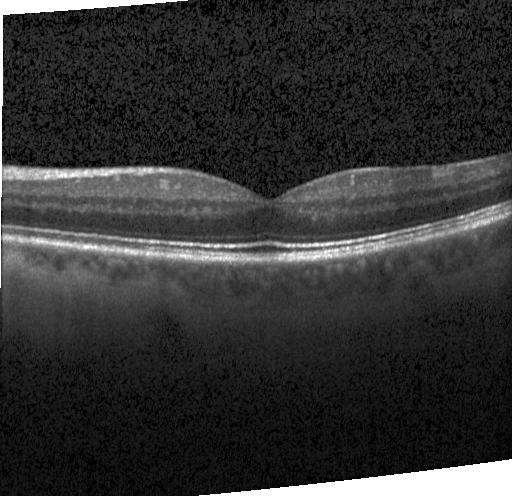

OCT line scan · Heidelberg Spectralis · horizontal scan through the fovea — Dx: no evidence of CNV, DME, or drusen.